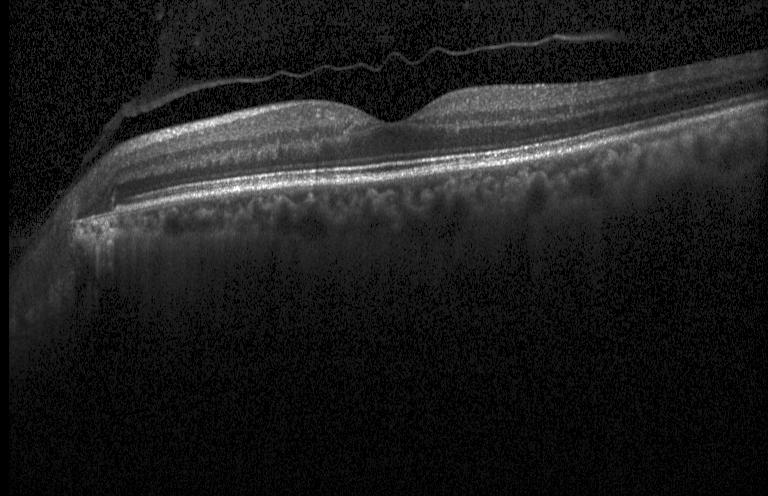

OCT line scan. Finding: no choroidal neovascularization, no diabetic macular edema, and no drusen.